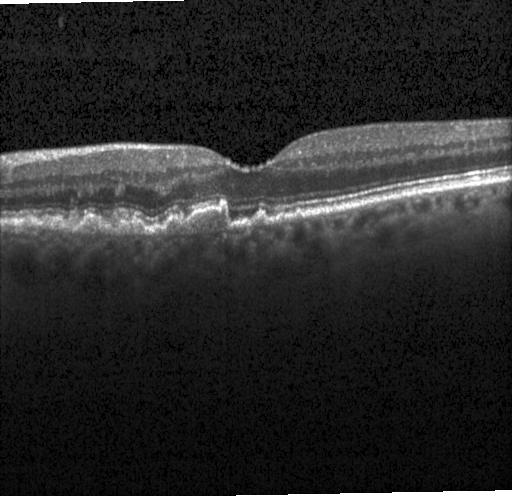
OCT line scan. Instrument: Heidelberg Spectralis. Fovea-centered — Assessment: drusen.